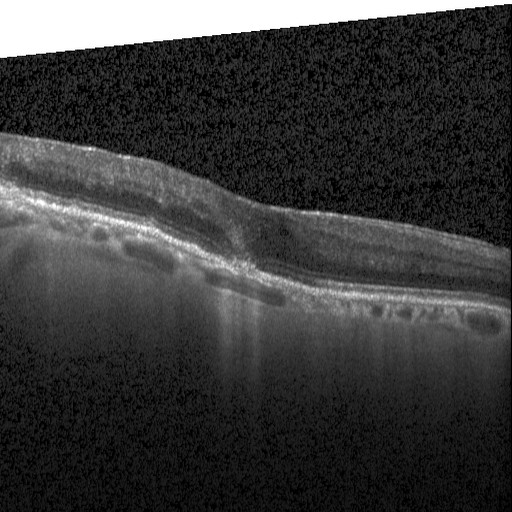
Spectral-domain OCT; retinal OCT B-scan.
Diagnosis: diabetic macular edema (DME).